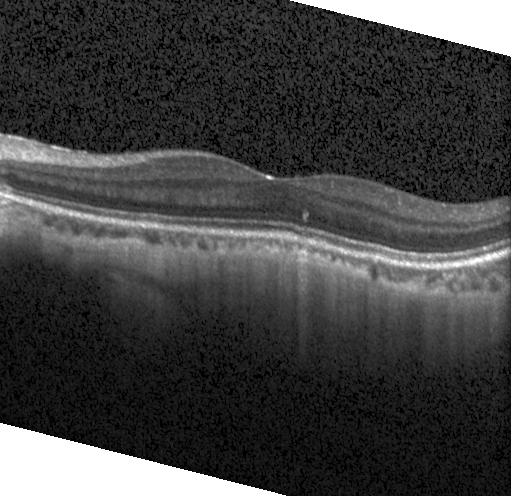
Retinal OCT cross-section; spectral-domain optical coherence tomography; instrument: Heidelberg Spectralis
Diagnosis: no CNV, DME, or drusen.